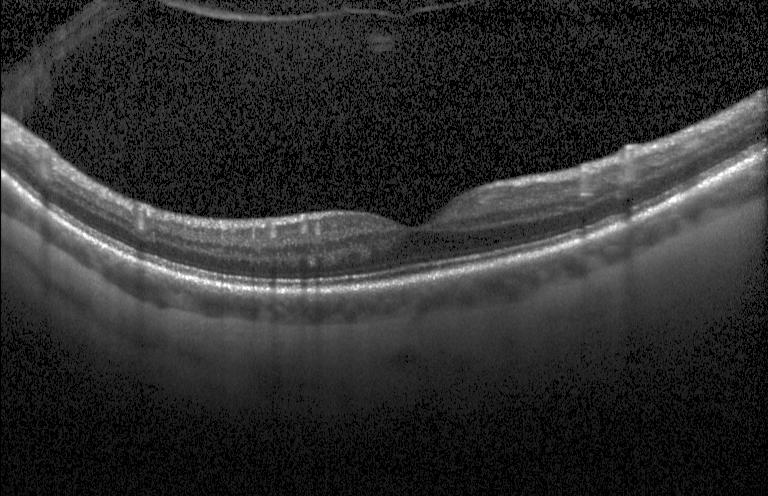

Retinal OCT cross-section
Diagnosis: no CNV, DME, or drusen.